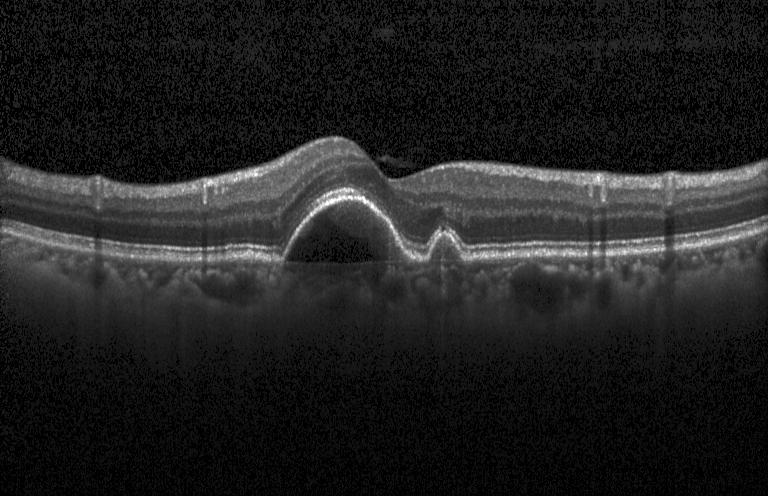

Finding: a choroidal neovascular membrane.